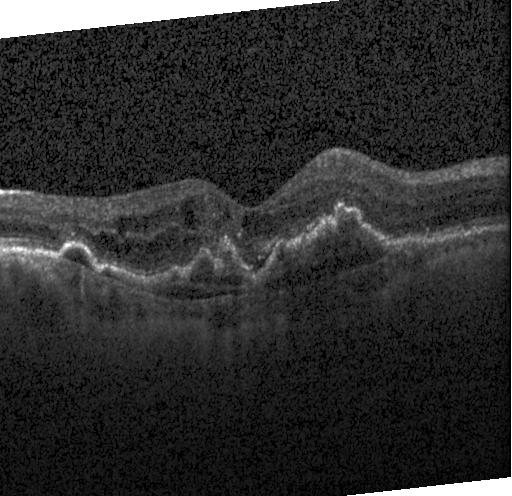 Through the macula. SD-OCT. Retinal OCT cross-section. A choroidal neovascular membrane.